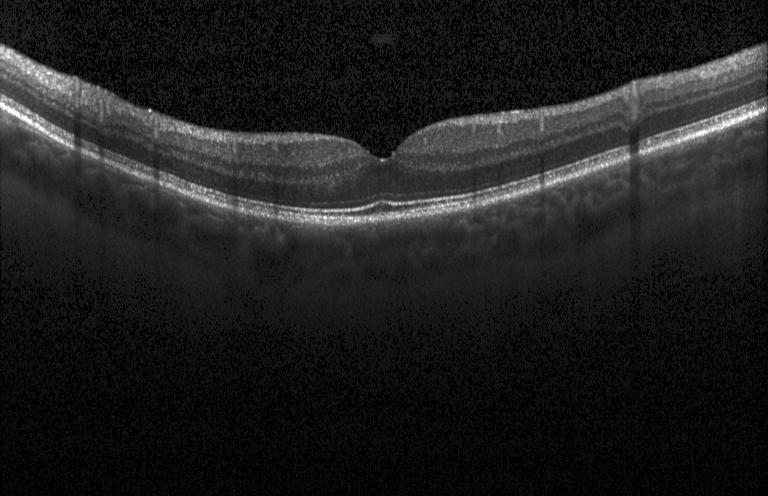
Retinal OCT cross-section showing no choroidal neovascularization, diabetic macular edema, or drusen.